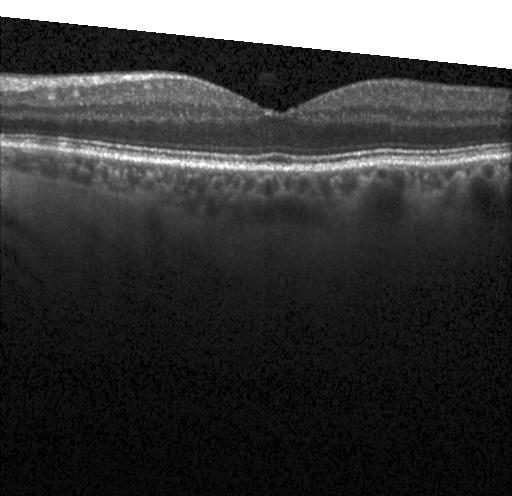
The scan shows no evidence of choroidal neovascularization, diabetic macular edema, or drusen.